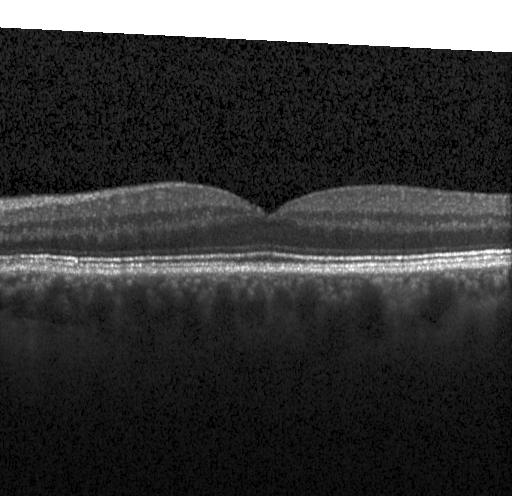
Macular scan; Heidelberg Spectralis; retinal OCT cross-section
Impression: no CNV, DME, or drusen.